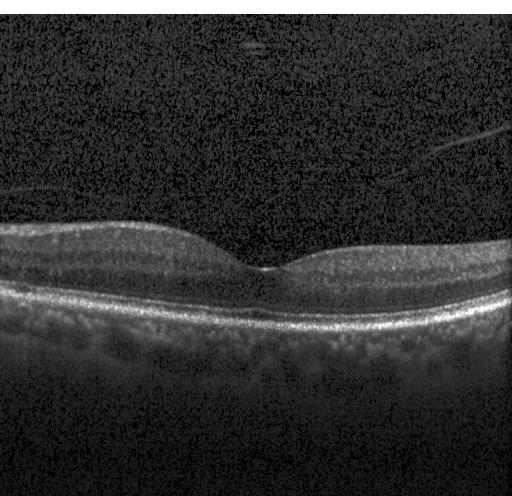 Retinal OCT cross-section, instrument: Heidelberg Spectralis, fovea-centered — Dx: neither choroidal neovascularization, diabetic macular edema, nor drusen.